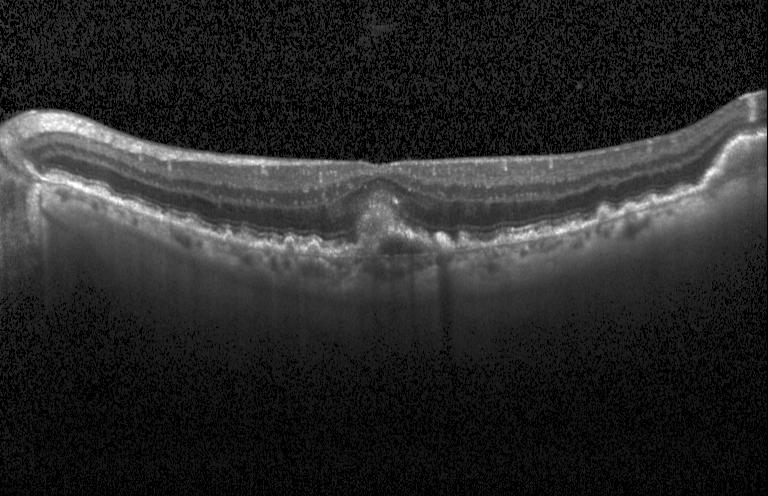
Retinal OCT B-scan — Dx: CNV.